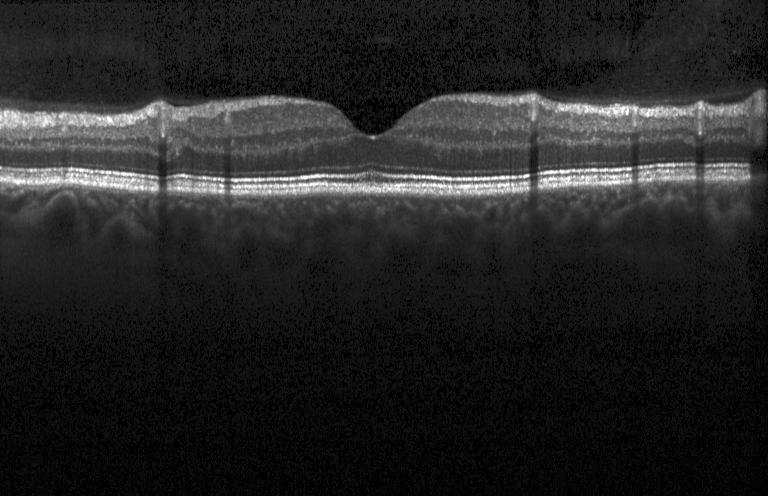 Retinal OCT cross-section · spectral-domain optical coherence tomography — Macular OCT: no choroidal neovascularization, diabetic macular edema, or drusen.